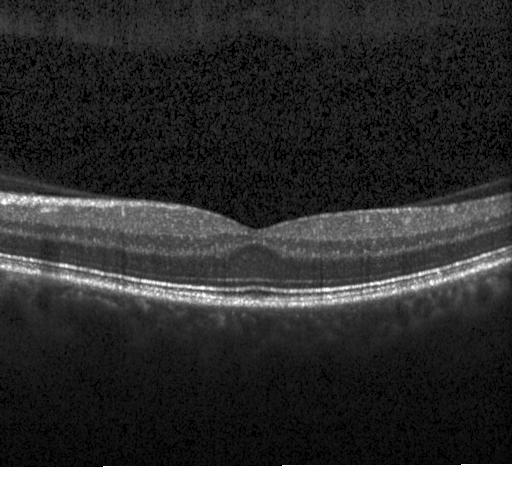

The scan shows no choroidal neovascularization, no diabetic macular edema, and no drusen.